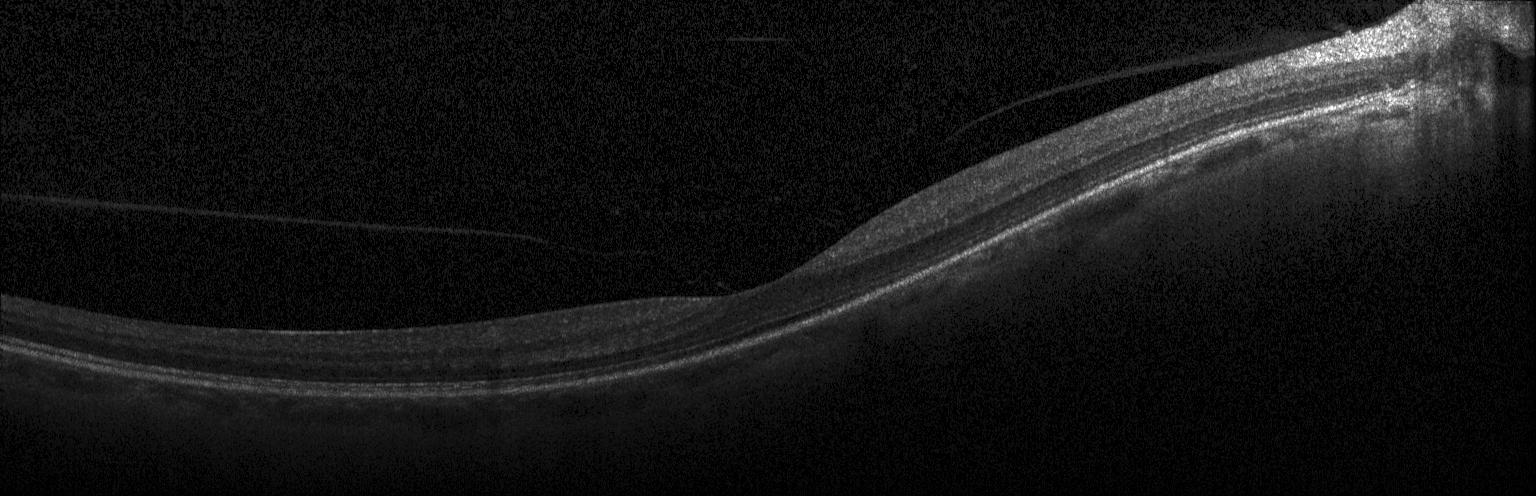
Instrument: Heidelberg Spectralis; retinal OCT B-scan — The scan shows no evidence of choroidal neovascularization, diabetic macular edema, or drusen.